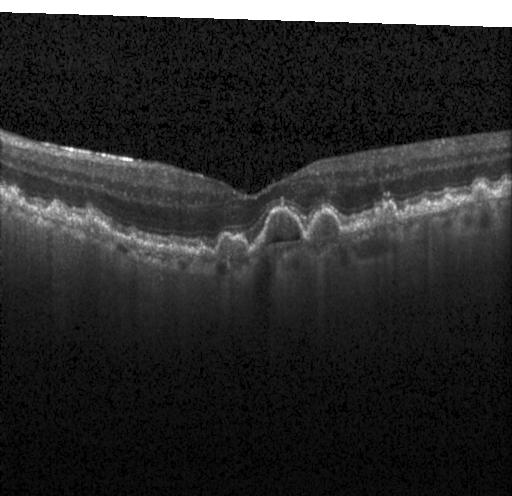
OCT B-scan
Impression: sub-RPE drusenoid deposits.